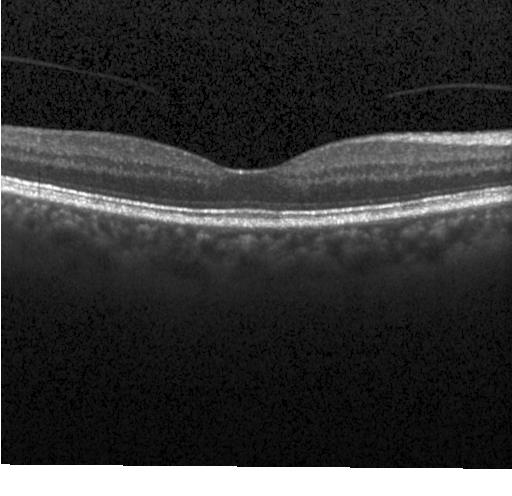 This B-scan demonstrates neither choroidal neovascularization, diabetic macular edema, nor drusen.